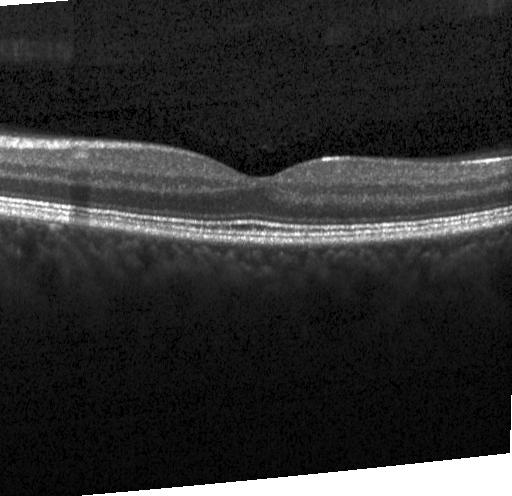
This B-scan demonstrates no choroidal neovascularization, diabetic macular edema, or drusen.